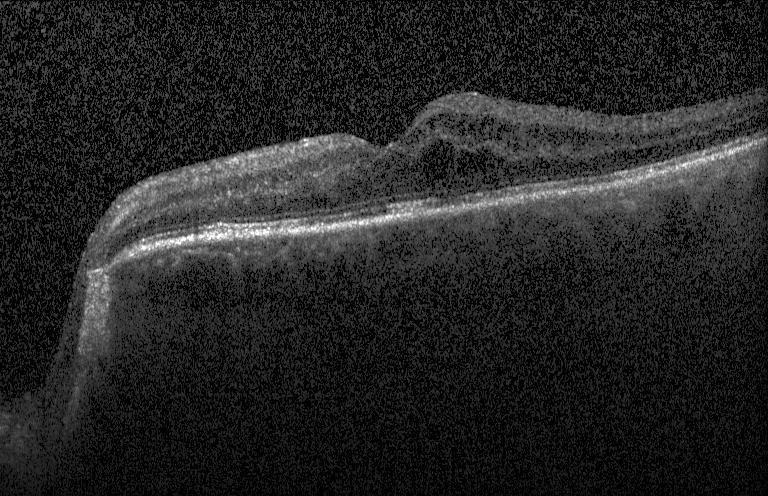
Optical coherence tomography scan
Finding: diabetic macular edema.